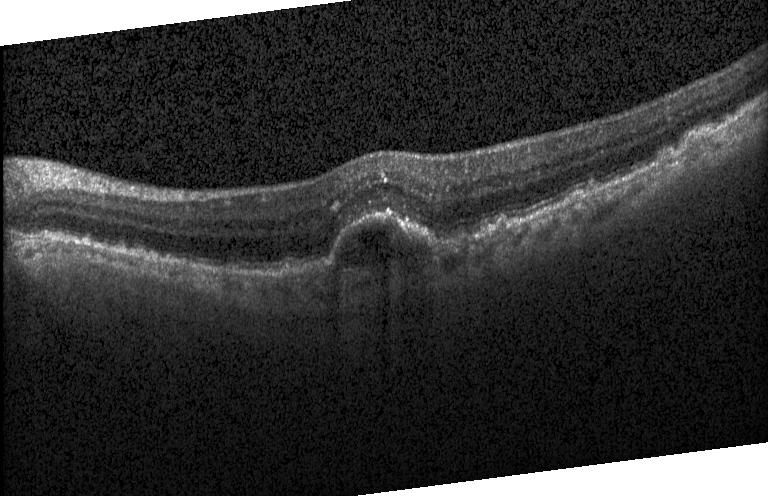 OCT B-scan; centered on the fovea; spectral-domain optical coherence tomography; Heidelberg Spectralis OCT system.
This B-scan demonstrates choroidal neovascularization (CNV).